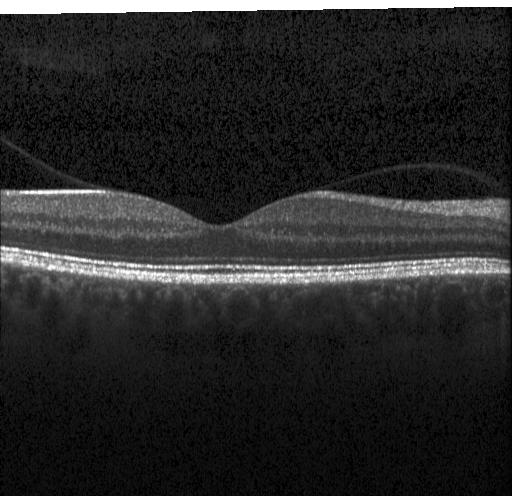
Spectral-domain optical coherence tomography · optical coherence tomography scan.
Finding: no evidence of choroidal neovascularization, diabetic macular edema, or drusen.